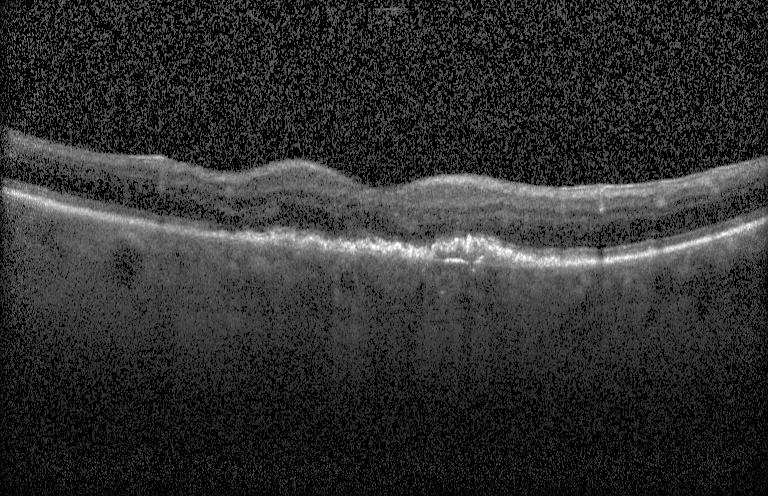
Optical coherence tomography scan — Finding: a choroidal neovascular membrane.